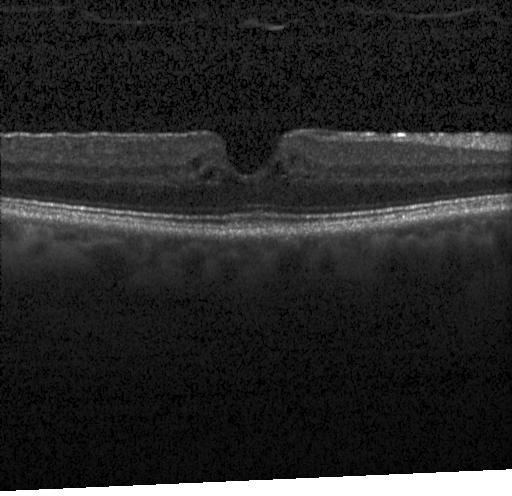 Retinal OCT cross-section · acquired on a Heidelberg Spectralis — This B-scan demonstrates diabetic macular edema (DME).